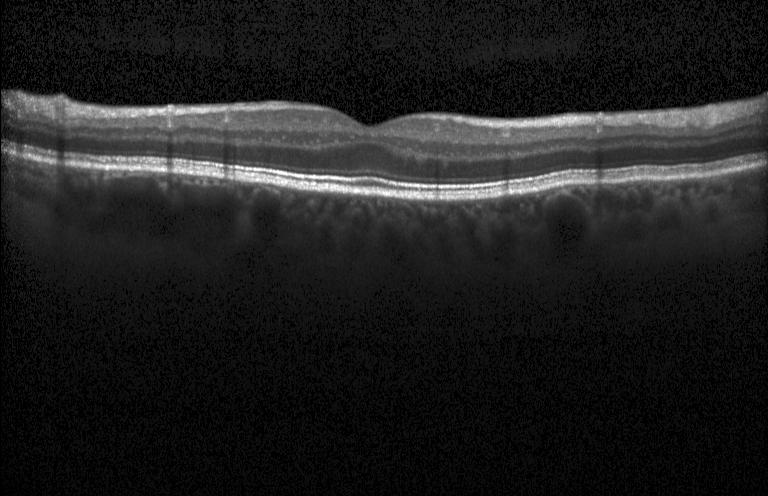

Heidelberg Spectralis. OCT B-scan. Centered on the fovea.
Diagnosis: no evidence of choroidal neovascularization, diabetic macular edema, or drusen.